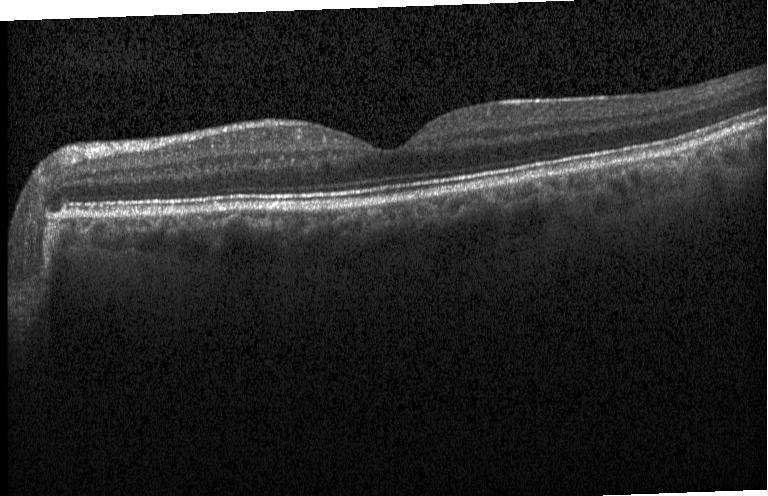

Impression: no CNV, DME, or drusen.